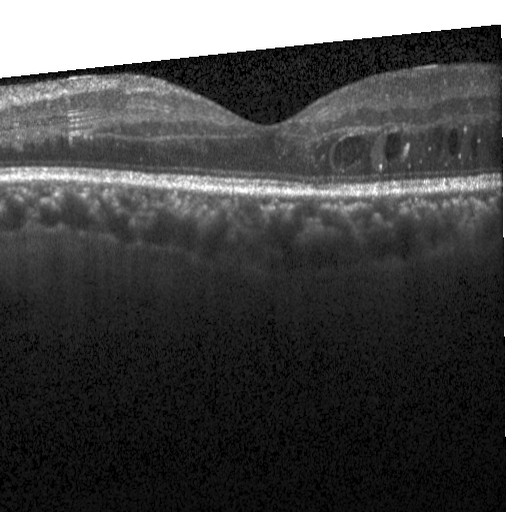

OCT B-scan · instrument: Heidelberg Spectralis — This B-scan demonstrates DME.